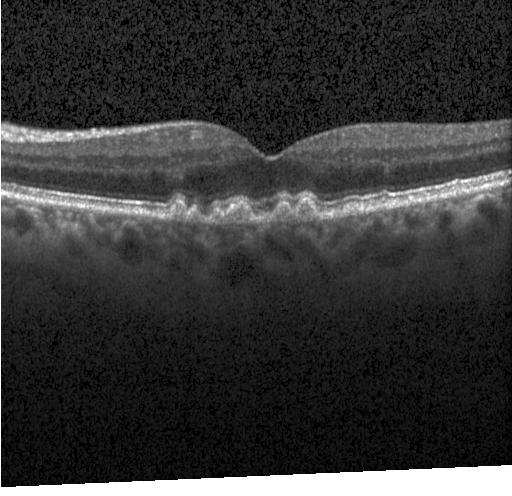 Retinal OCT B-scan. Spectral-domain OCT.
Dx: multiple drusen.